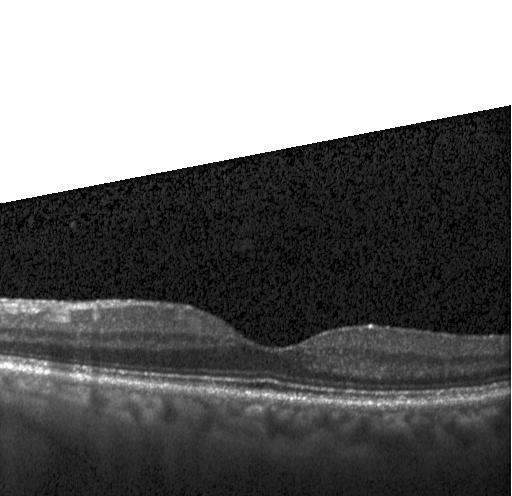
Retinal OCT cross-section showing no evidence of choroidal neovascularization, diabetic macular edema, or drusen.